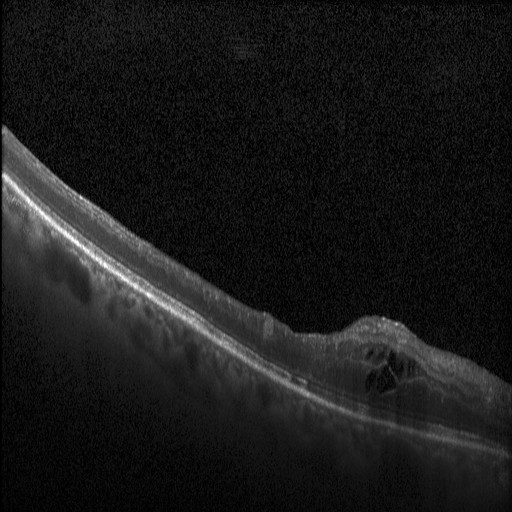

OCT B-scan showing diabetic macular edema (DME).